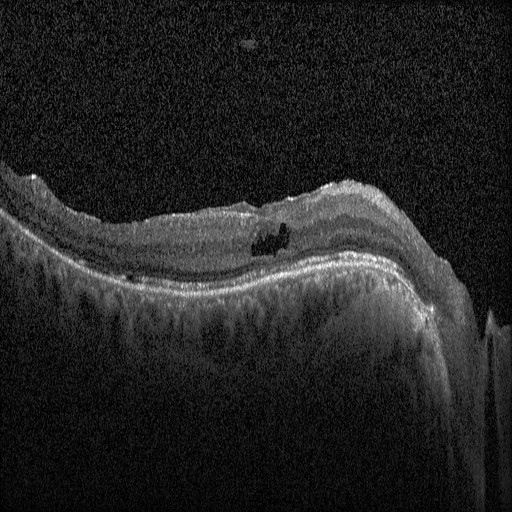 Spectral-domain optical coherence tomography; optical coherence tomography scan; Heidelberg Spectralis; through the macula — This B-scan demonstrates diabetic macular edema (DME).